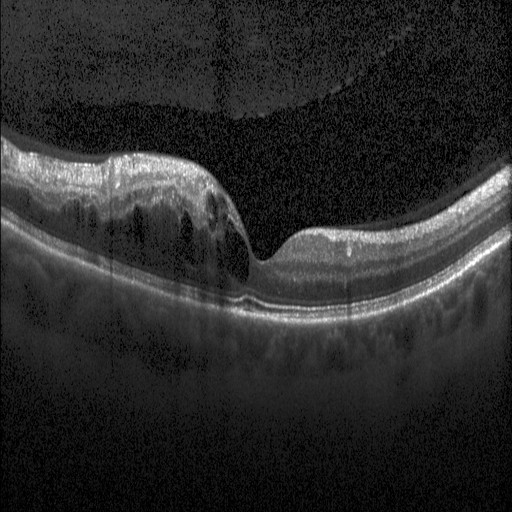

Retinal OCT cross-section.
Assessment: DME.